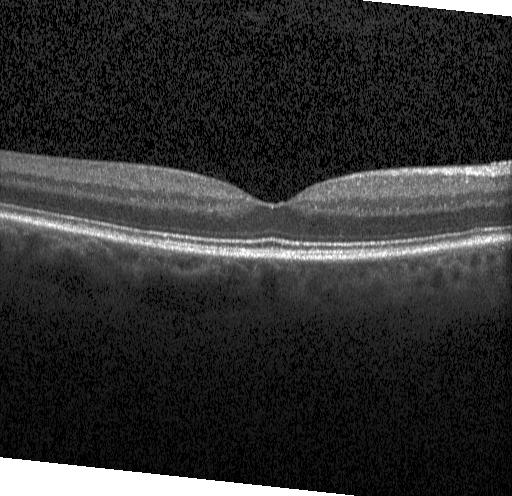 Impression: no evidence of choroidal neovascularization, diabetic macular edema, or drusen.